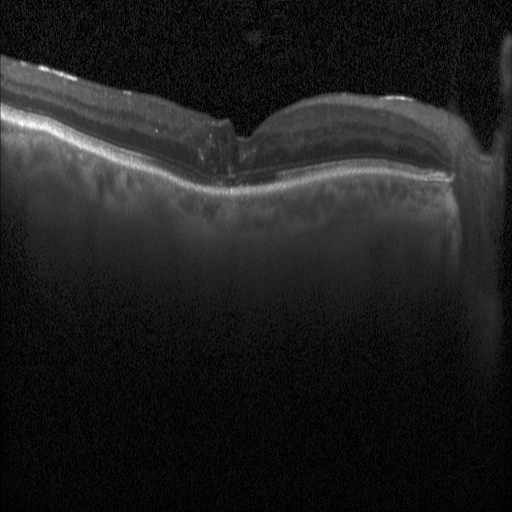
Instrument: Heidelberg Spectralis, optical coherence tomography B-scan.
Impression: DME.